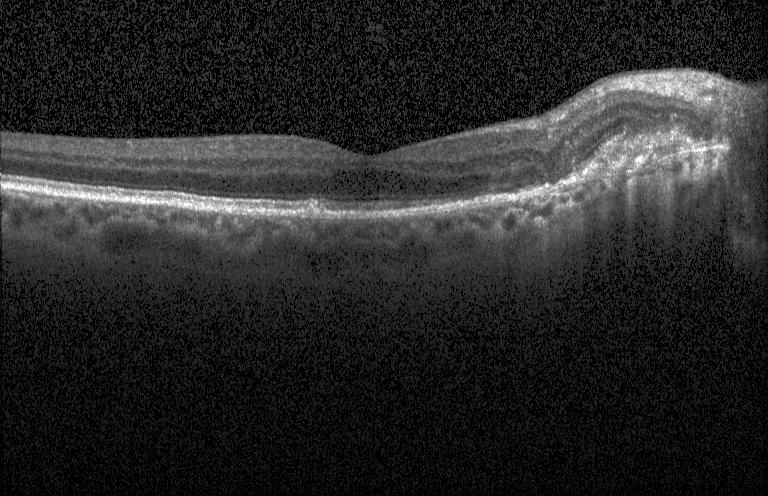
Macular OCT: choroidal neovascularization (CNV).